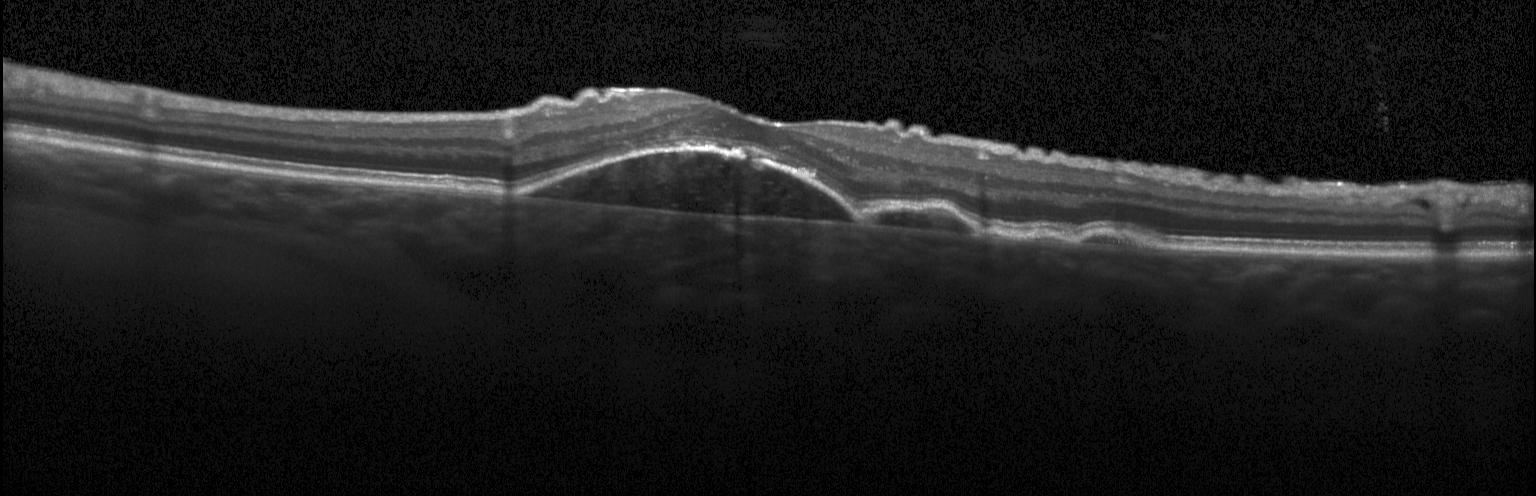 Retinal OCT cross-section · spectral-domain OCT — Diagnosis: choroidal neovascularization.